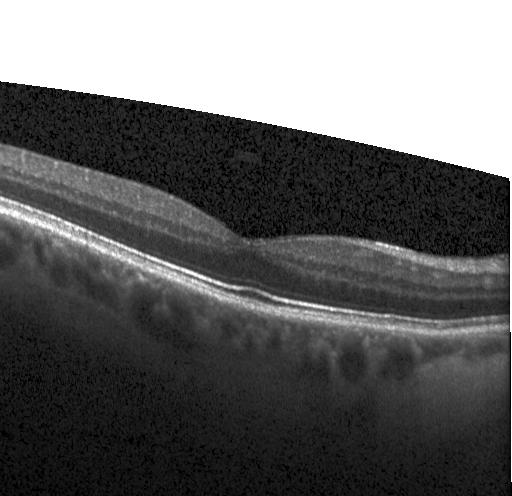 Instrument: Heidelberg Spectralis. Retinal OCT cross-section. Through the macula. SD-OCT. Impression: neither choroidal neovascularization, diabetic macular edema, nor drusen.